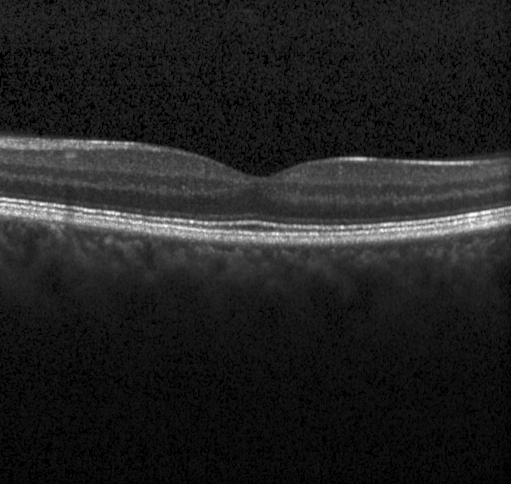

Retinal OCT B-scan.
Diagnosis: no choroidal neovascularization, diabetic macular edema, or drusen.